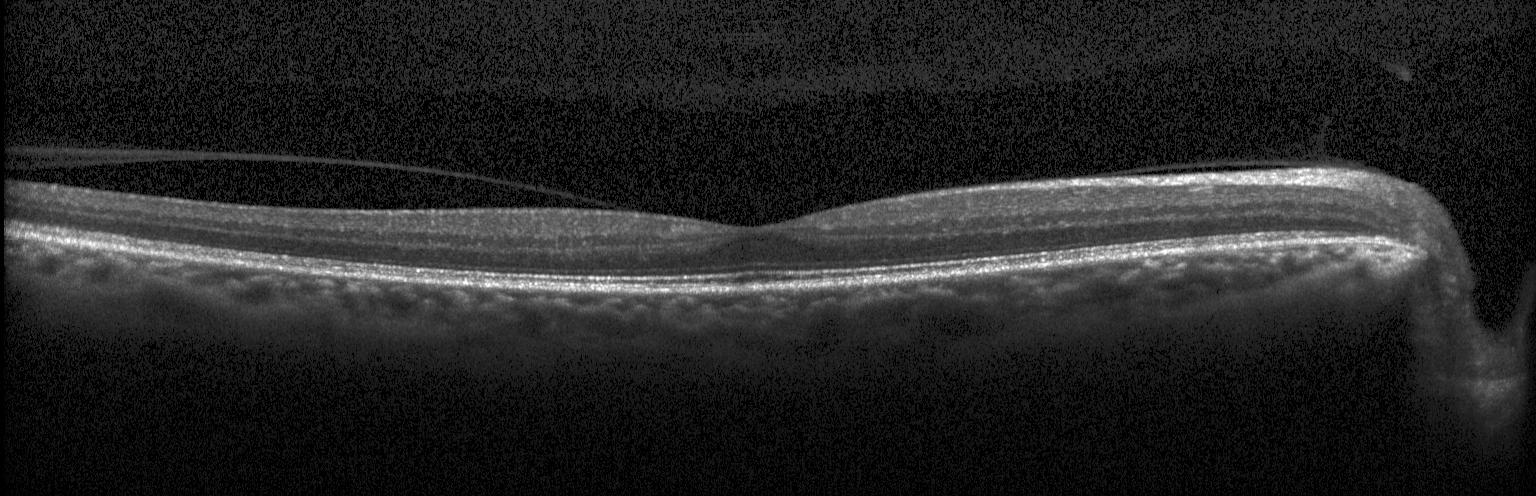 Heidelberg Spectralis; optical coherence tomography B-scan; spectral-domain optical coherence tomography — The scan shows no CNV, no DME, and no drusen.